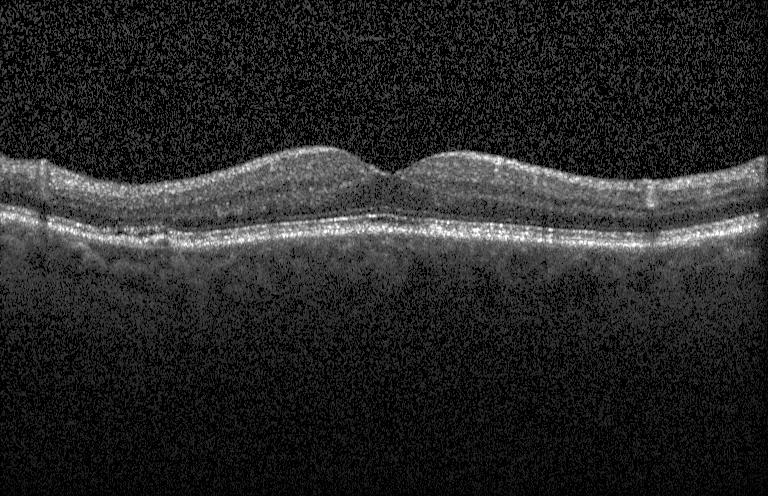 Horizontal scan through the fovea. OCT B-scan — This B-scan demonstrates a choroidal neovascular membrane.